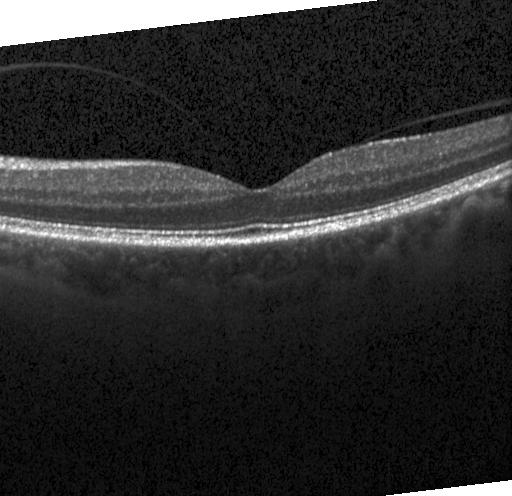

Retinal OCT cross-section · fovea-centered · SD-OCT · acquired on a Heidelberg Spectralis
Assessment: no choroidal neovascularization, diabetic macular edema, or drusen.